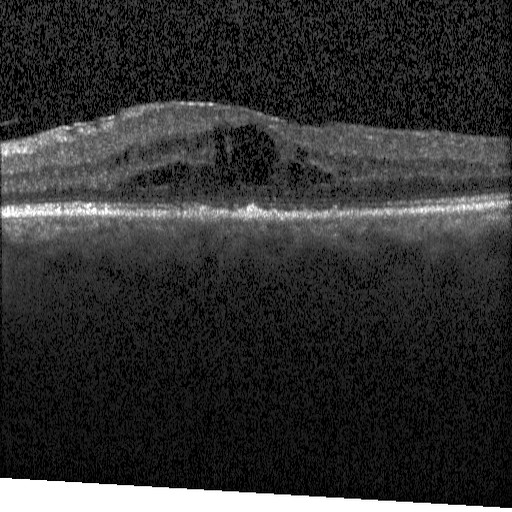

Through the macula; OCT B-scan. Assessment: diabetic macular edema.